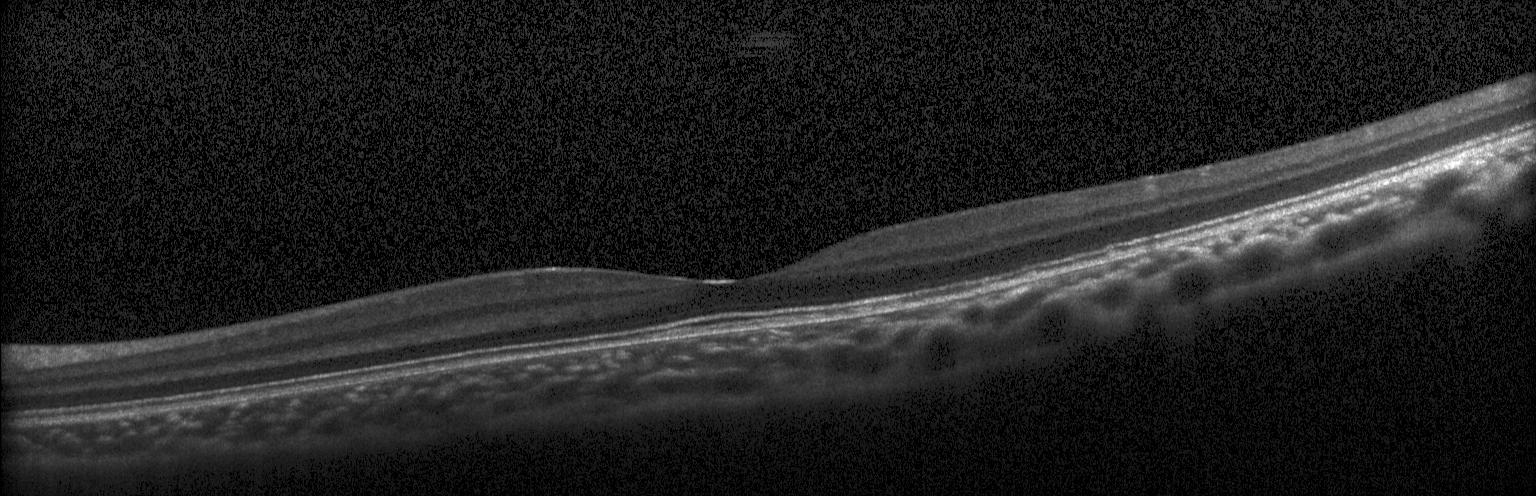

Macular OCT demonstrating no CNV, no DME, and no drusen.